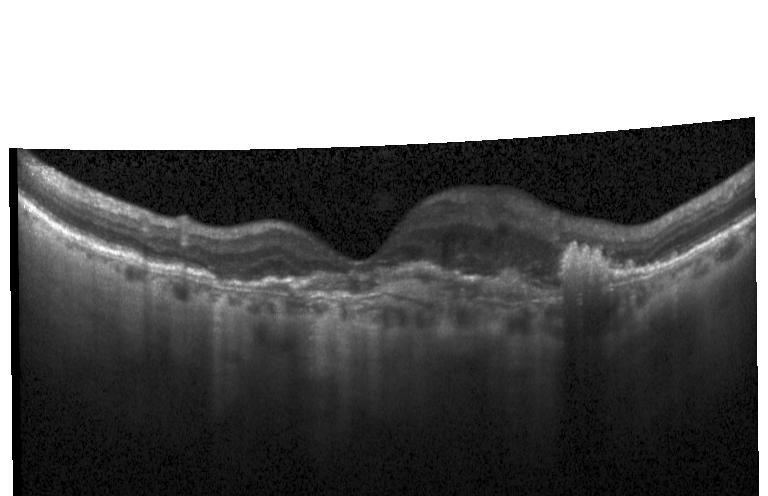
Instrument: Heidelberg Spectralis; OCT line scan; spectral-domain OCT
Impression: choroidal neovascularization (CNV).